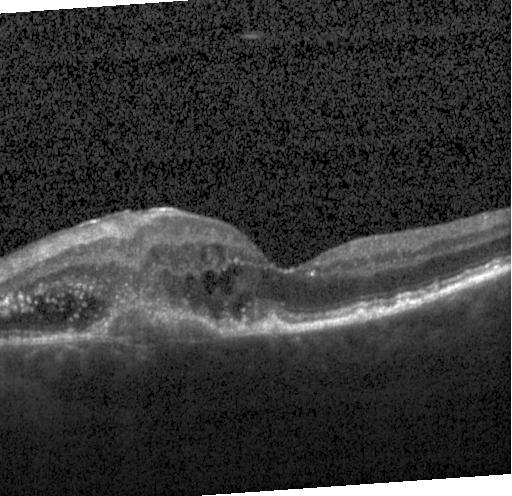

Through the macula. OCT B-scan — OCT finding: a choroidal neovascular membrane.